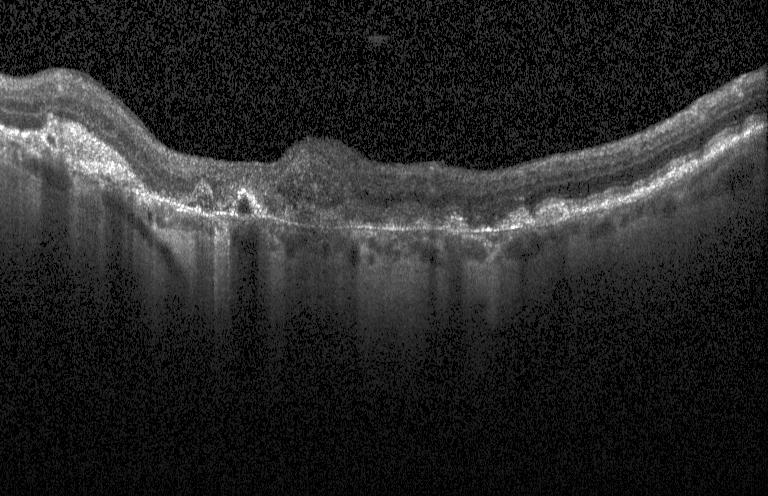

Dx: a choroidal neovascular membrane.